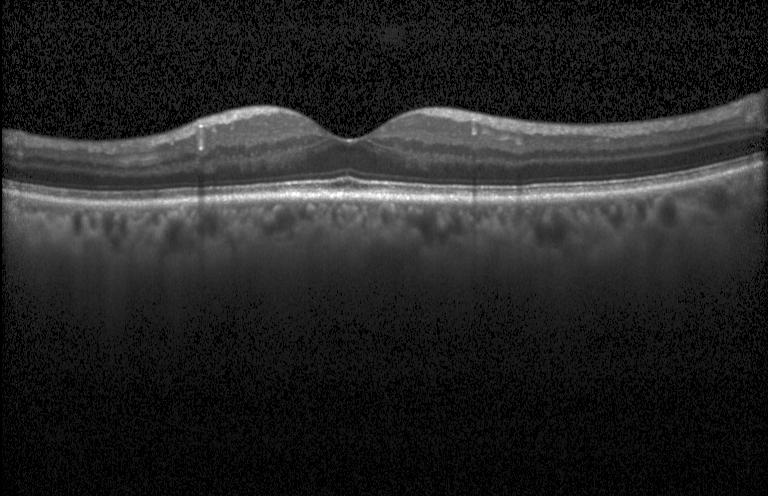 Retinal OCT B-scan · spectral-domain optical coherence tomography — Macular OCT: neither CNV, DME, nor drusen.